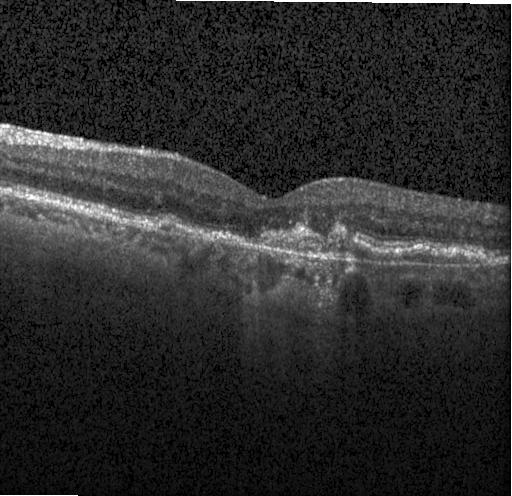 This B-scan demonstrates a choroidal neovascular membrane.